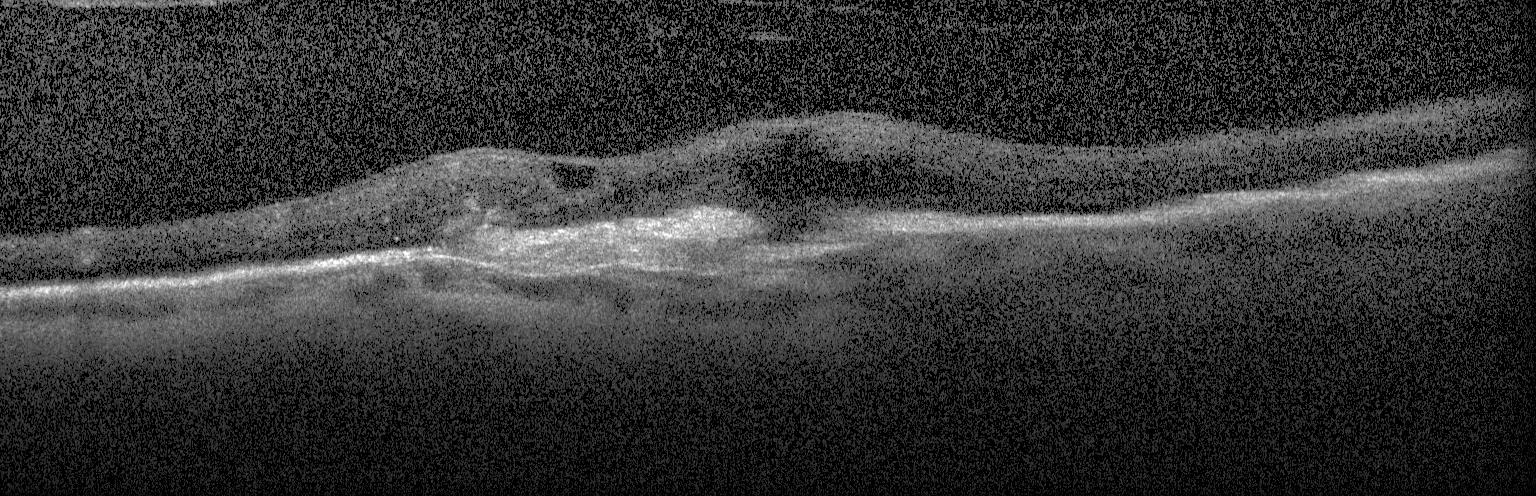
OCT finding: choroidal neovascularization (CNV).